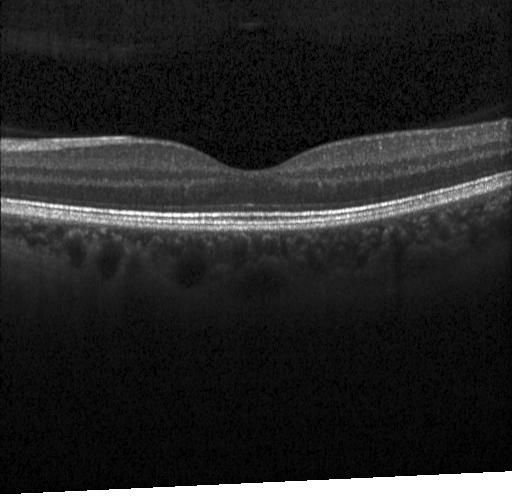
OCT line scan; fovea-centered; acquired on a Heidelberg Spectralis.
Impression: no evidence of choroidal neovascularization, diabetic macular edema, or drusen.